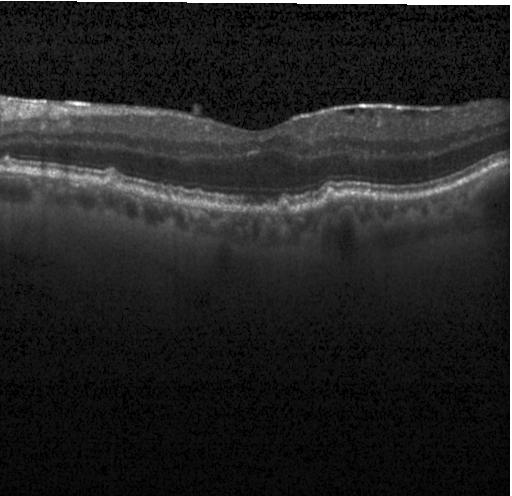

Optical coherence tomography B-scan — Diagnosis: sub-RPE drusenoid deposits.